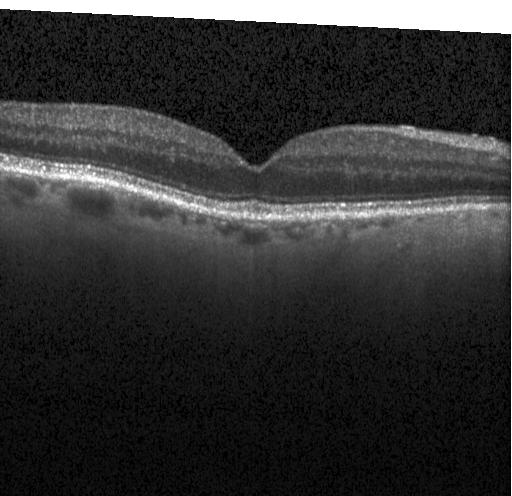 The scan shows no choroidal neovascularization, no diabetic macular edema, and no drusen.